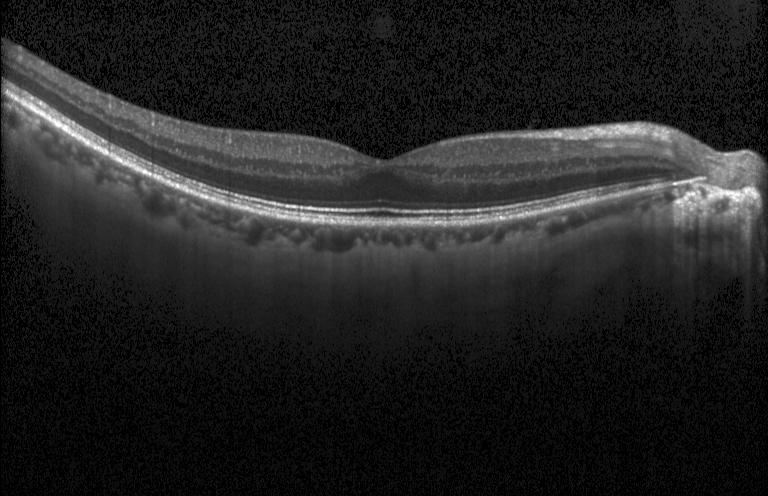 Optical coherence tomography scan — This B-scan demonstrates neither choroidal neovascularization, diabetic macular edema, nor drusen.